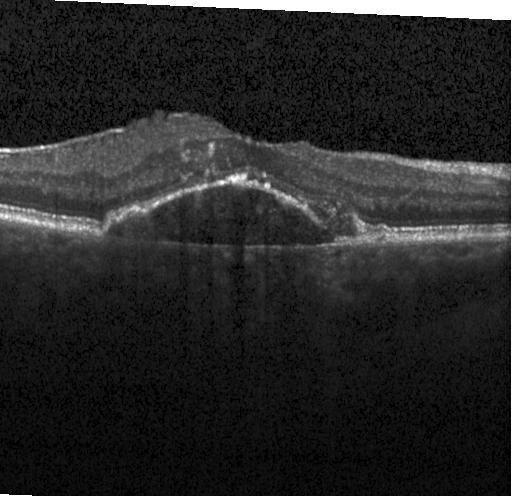
Finding: choroidal neovascularization.